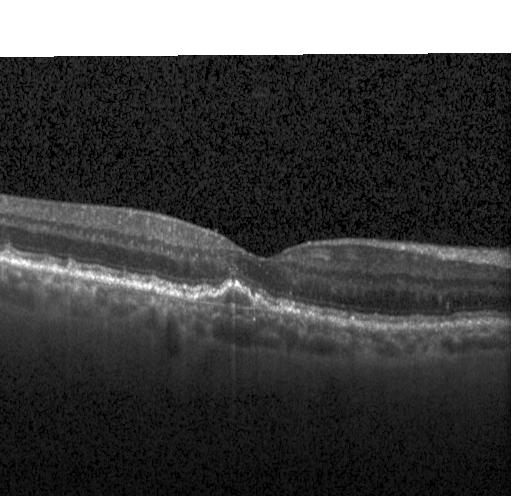 Optical coherence tomography B-scan — Finding: choroidal neovascularization.